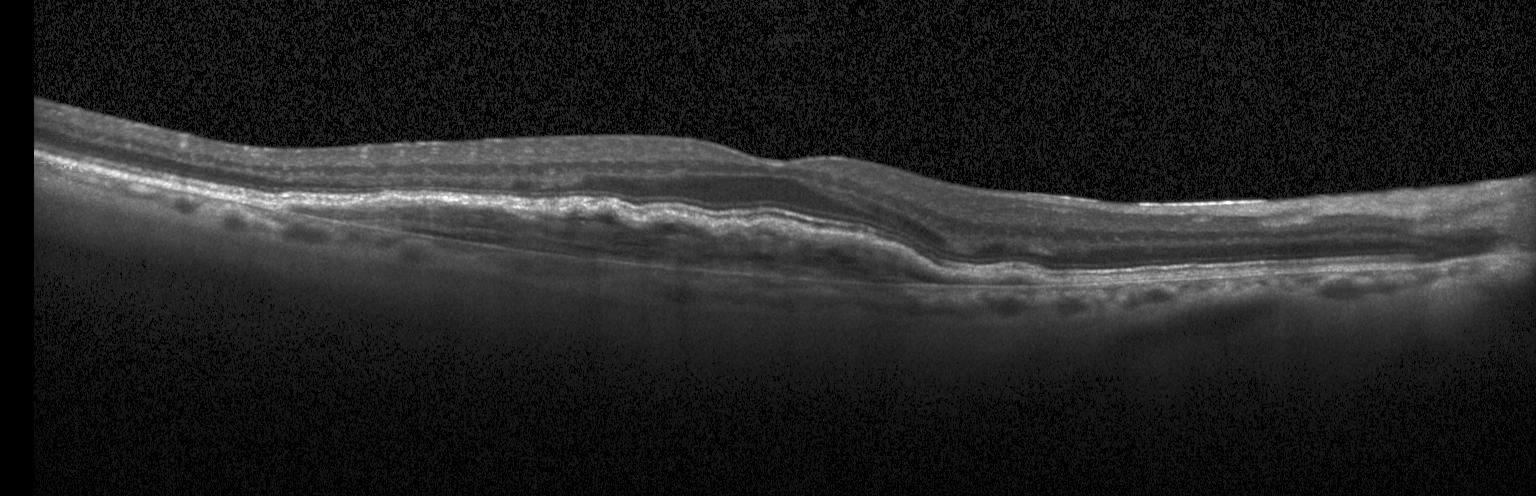

Retinal OCT cross-section — Impression: a choroidal neovascular membrane.